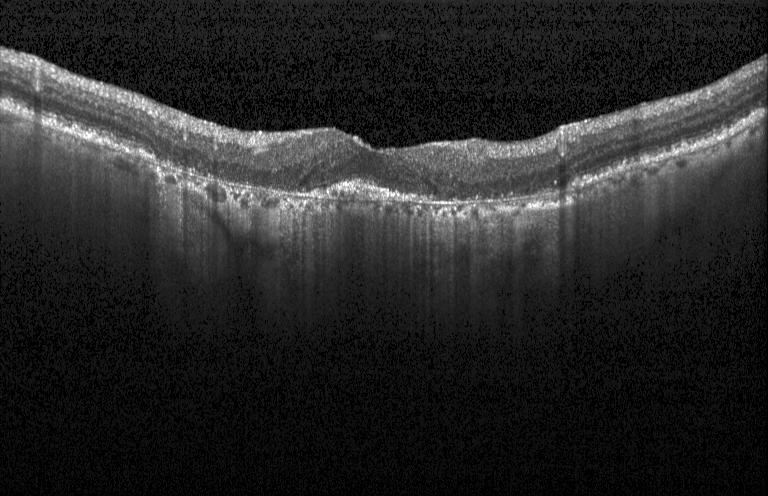

OCT B-scan — Impression: choroidal neovascularization (CNV).